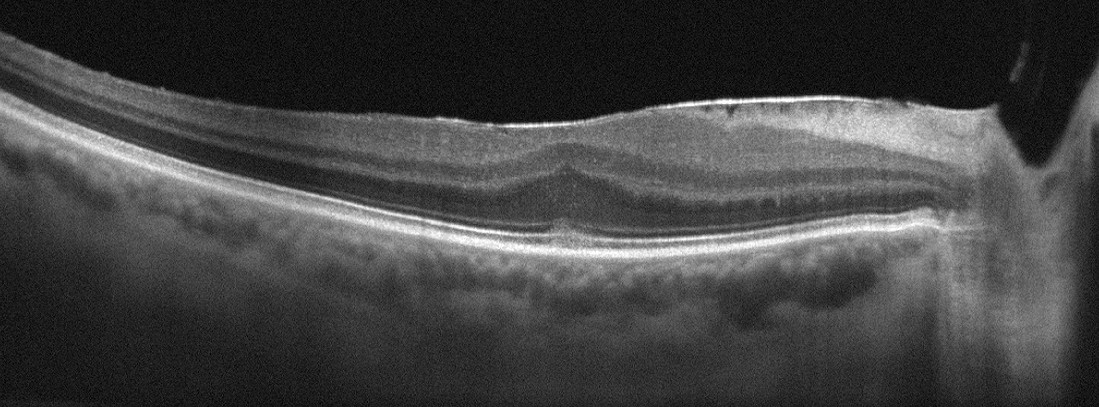
Optovue Avanti RTVue XR, optical coherence tomography scan
Dx: ERM.